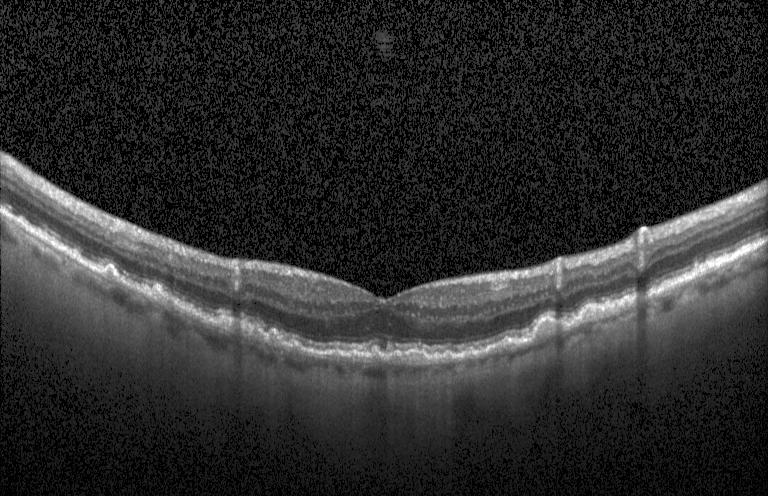 Impression: sub-RPE drusenoid deposits.